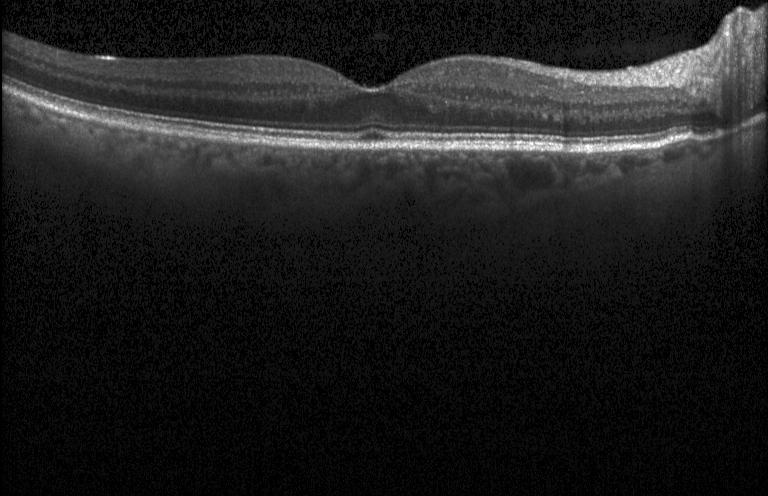
Optical coherence tomography scan — Finding: no evidence of CNV, DME, or drusen.